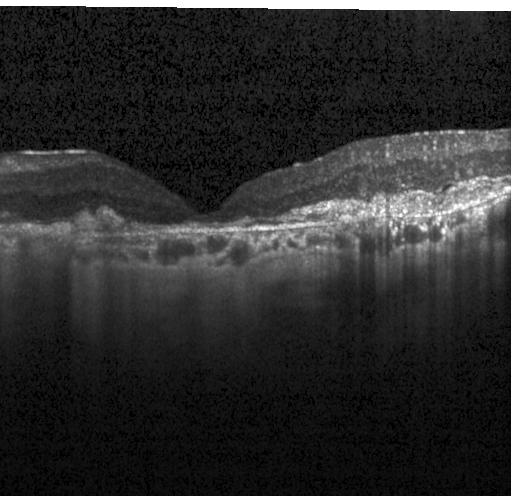 Retinal OCT cross-section showing CNV.